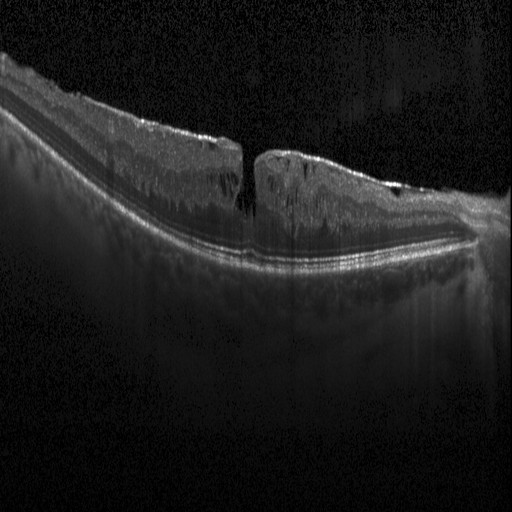
Macular scan, SD-OCT, Heidelberg Spectralis, optical coherence tomography B-scan. Impression: diabetic macular edema (DME).